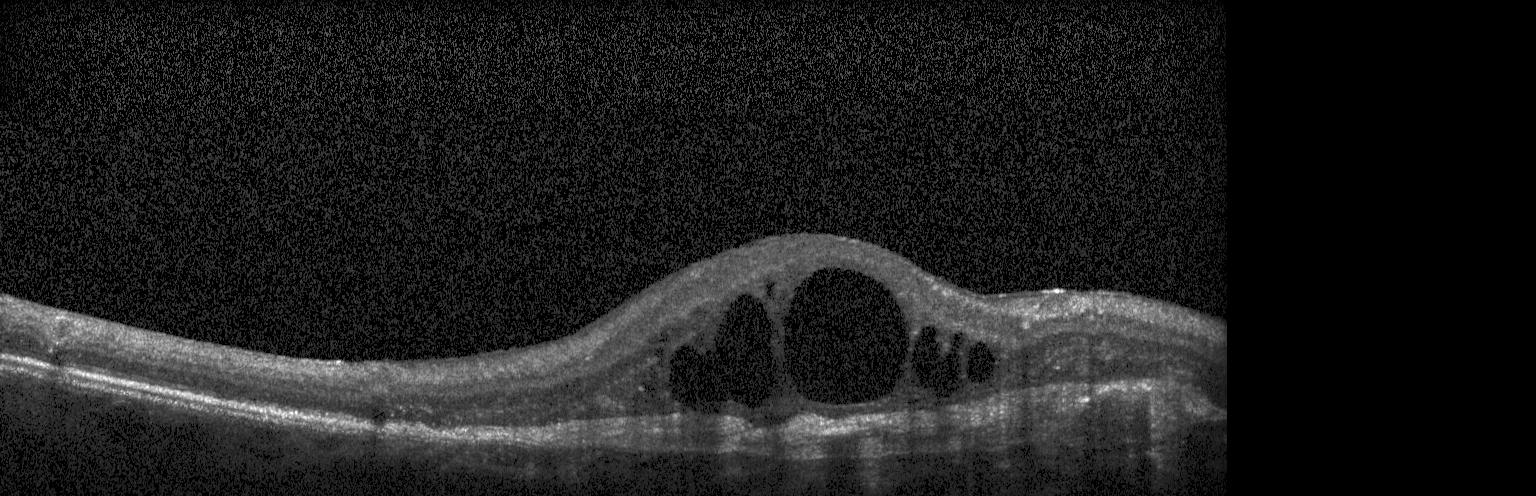

Optical coherence tomography B-scan · spectral-domain optical coherence tomography — A choroidal neovascular membrane.